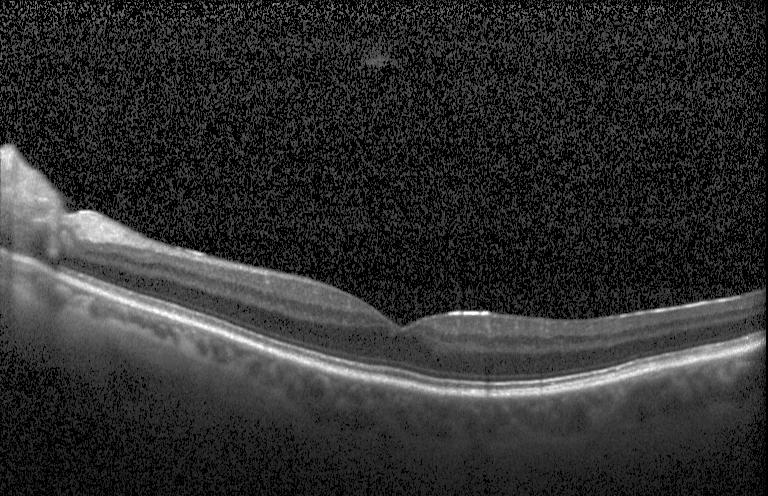
Instrument: Heidelberg Spectralis, optical coherence tomography B-scan, spectral-domain OCT.
The scan shows no CNV, no DME, and no drusen.